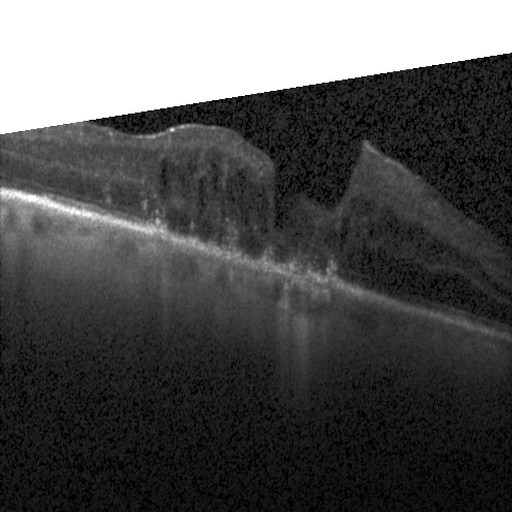

Retinal OCT cross-section — This B-scan demonstrates DME.